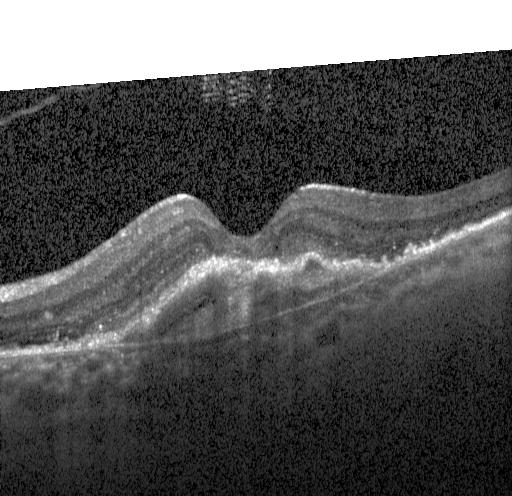
Impression: CNV.